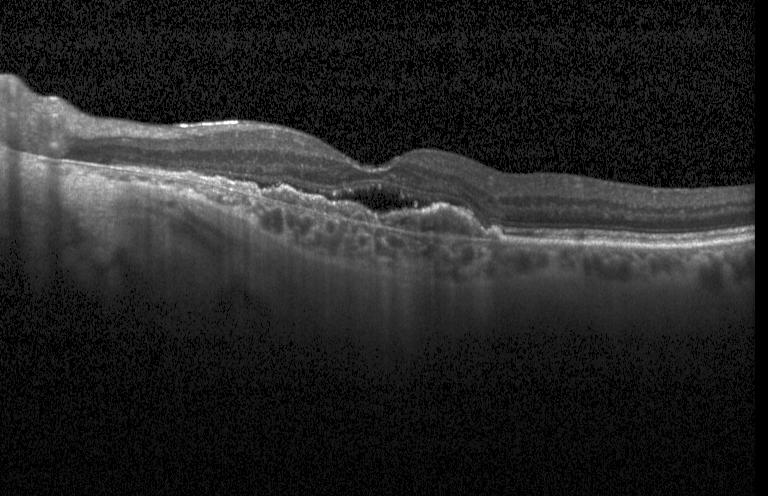 Fovea-centered · SD-OCT · OCT B-scan · instrument: Heidelberg Spectralis. Diagnosis: CNV.